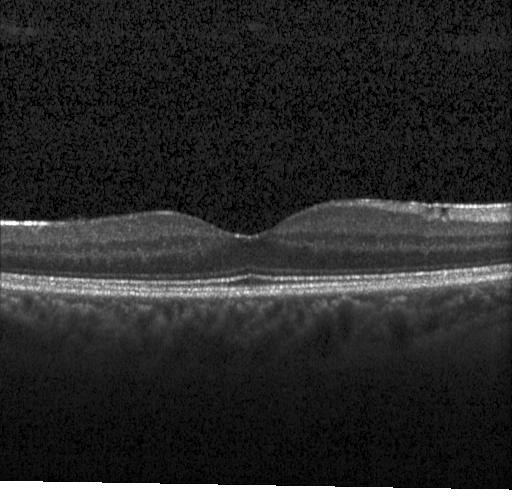

Impression: no choroidal neovascularization, diabetic macular edema, or drusen.